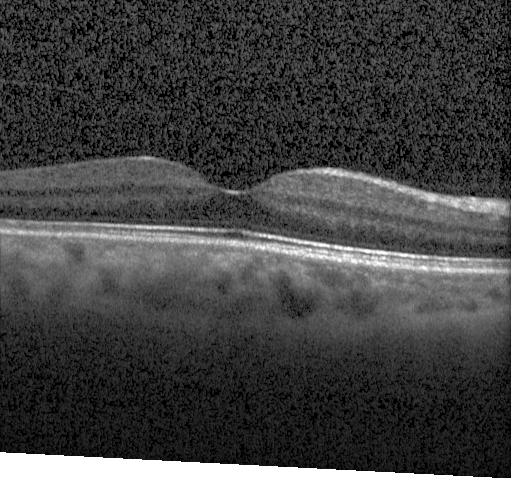

Spectral-domain OCT · OCT B-scan — Assessment: no choroidal neovascularization, no diabetic macular edema, and no drusen.